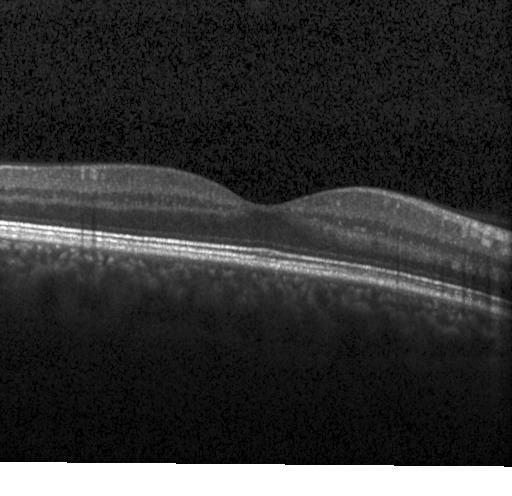 Centered on the fovea, retinal OCT cross-section.
Diagnosis: no choroidal neovascularization, diabetic macular edema, or drusen.